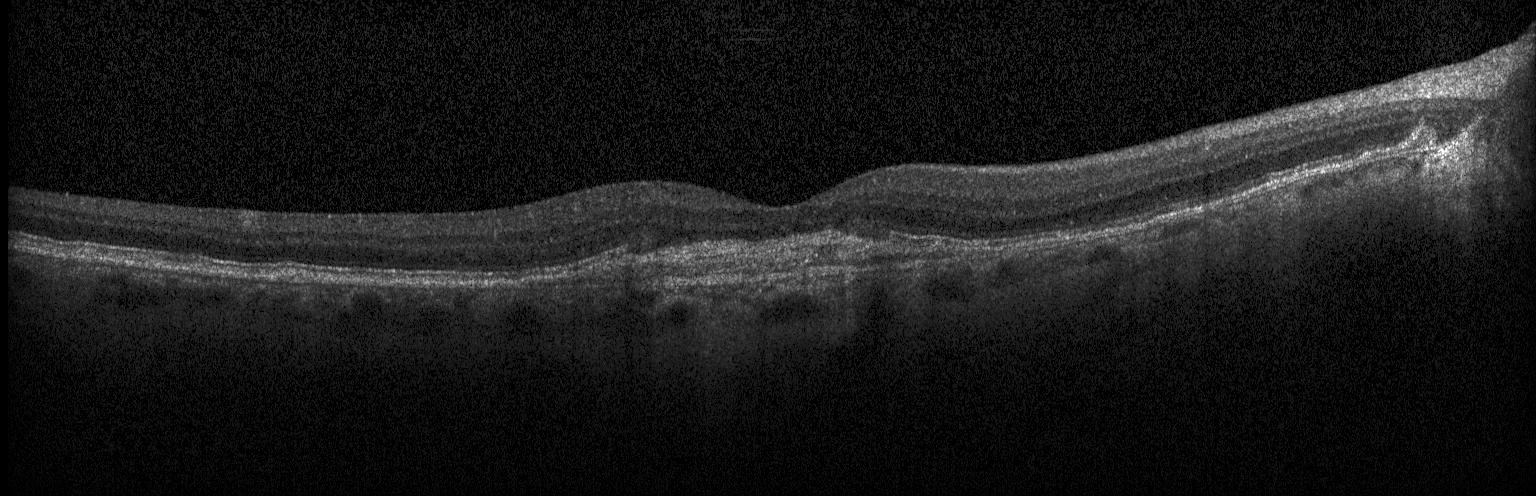
Assessment: choroidal neovascularization (CNV).